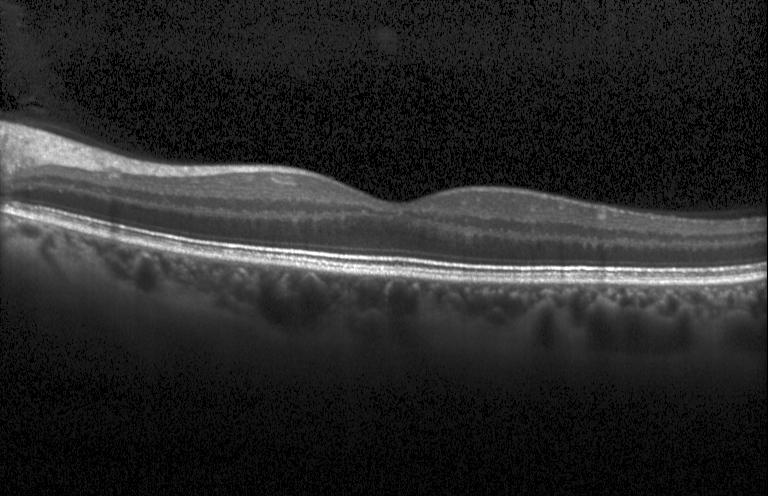

Horizontal scan through the fovea. Acquired on a Heidelberg Spectralis. OCT line scan
Impression: neither choroidal neovascularization, diabetic macular edema, nor drusen.